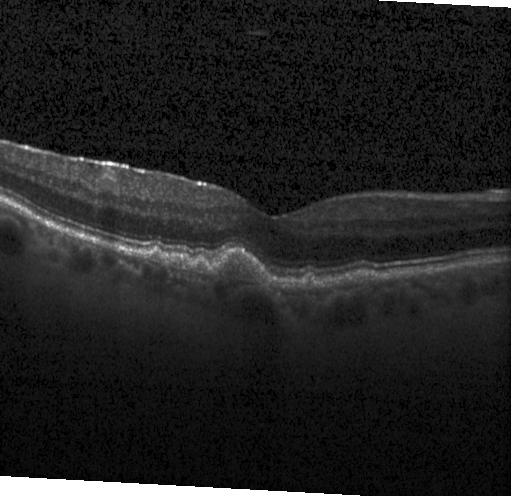

Fovea-centered. OCT B-scan. Heidelberg Spectralis.
Finding: drusen.